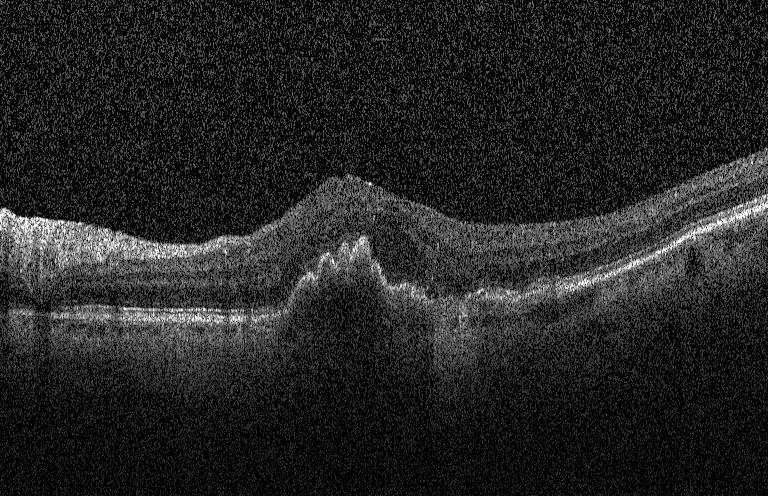

Diagnosis: a choroidal neovascular membrane.